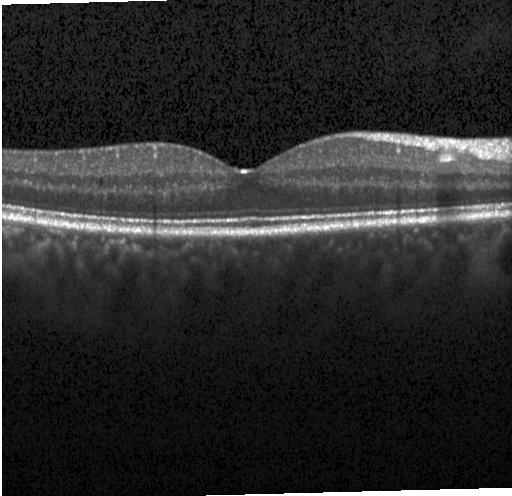 Spectral-domain optical coherence tomography; Heidelberg Spectralis; retinal OCT B-scan; horizontal scan through the fovea
Macular OCT: neither CNV, DME, nor drusen.